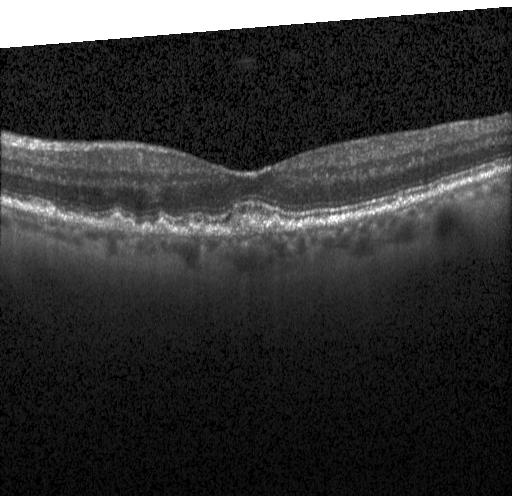
Retinal OCT cross-section
Finding: multiple drusen.